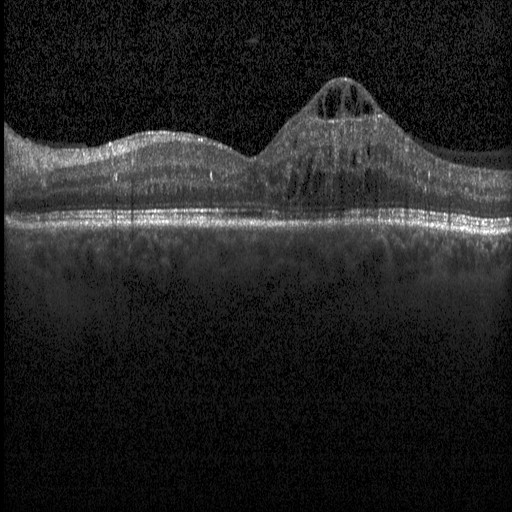
Heidelberg Spectralis OCT system. Optical coherence tomography B-scan
Diagnosis: diabetic macular edema (DME).